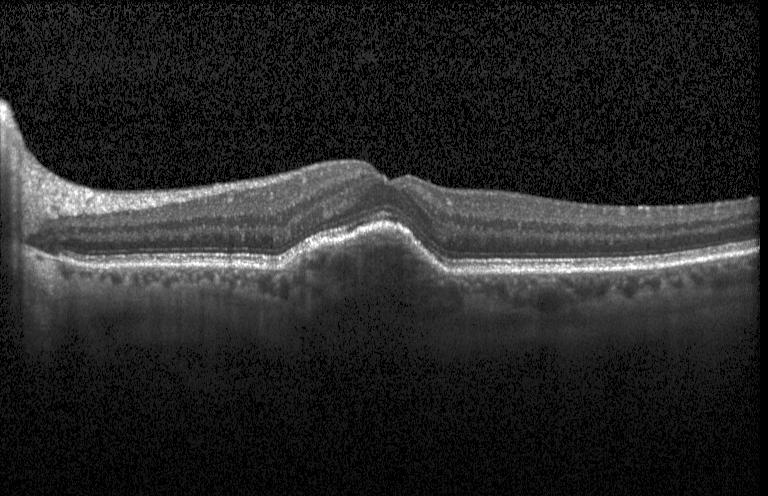
Choroidal neovascularization (CNV).